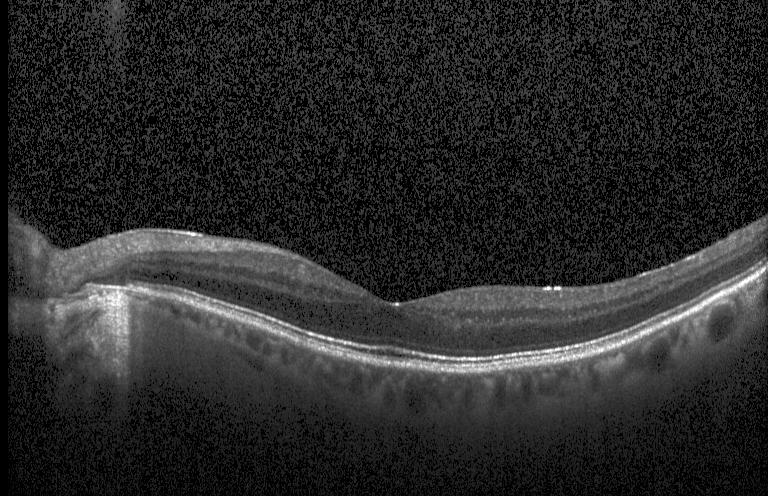

OCT B-scan · centered on the fovea · Heidelberg Spectralis OCT system · SD-OCT
No CNV, no DME, and no drusen.